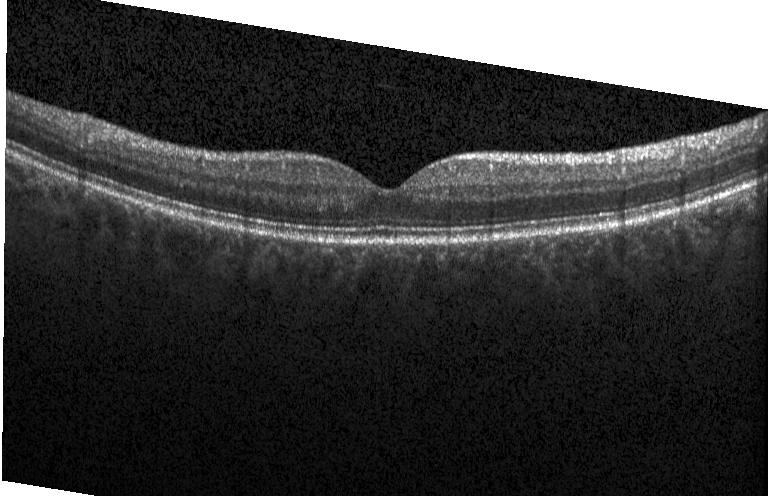 Spectral-domain OCT · OCT line scan. Impression: no evidence of CNV, DME, or drusen.